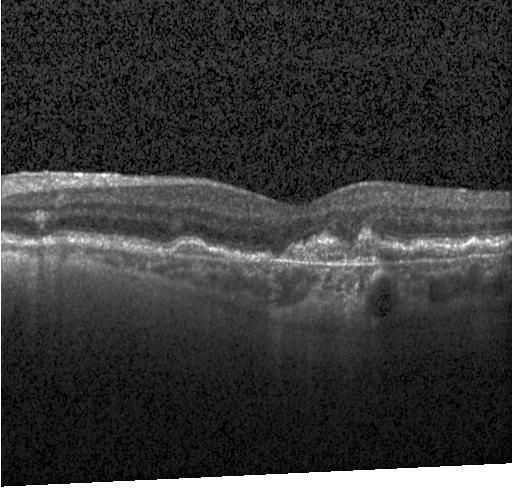

Optical coherence tomography B-scan.
Impression: a choroidal neovascular membrane.